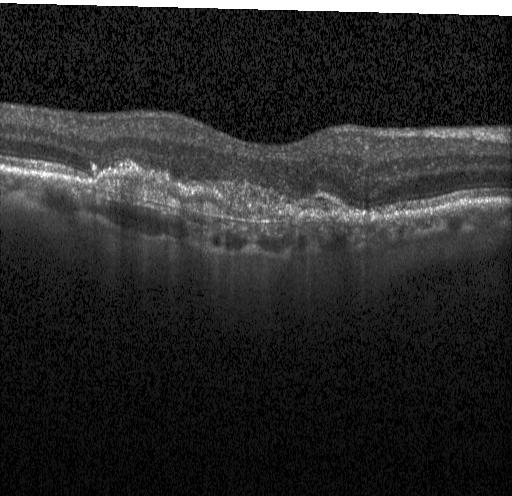
Heidelberg Spectralis OCT system. Optical coherence tomography B-scan. SD-OCT
OCT finding: a choroidal neovascular membrane.